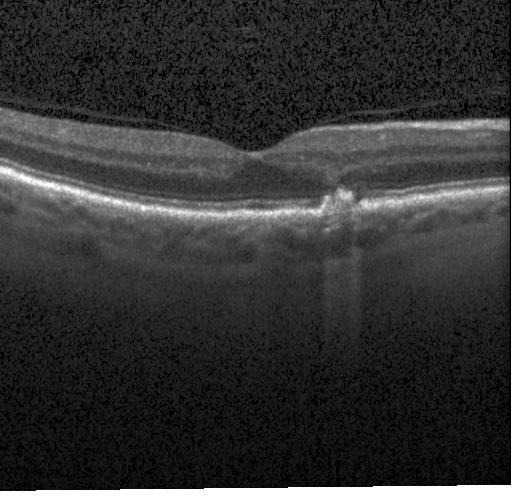
Spectral-domain optical coherence tomography. Retinal OCT cross-section. Acquired on a Heidelberg Spectralis
OCT finding: drusen.